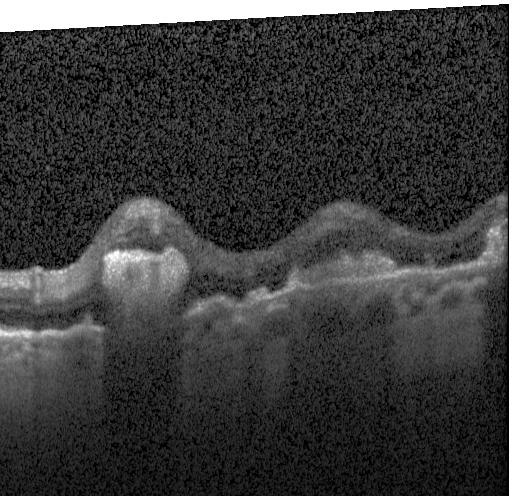
Fovea-centered; SD-OCT; OCT line scan.
Dx: a choroidal neovascular membrane.